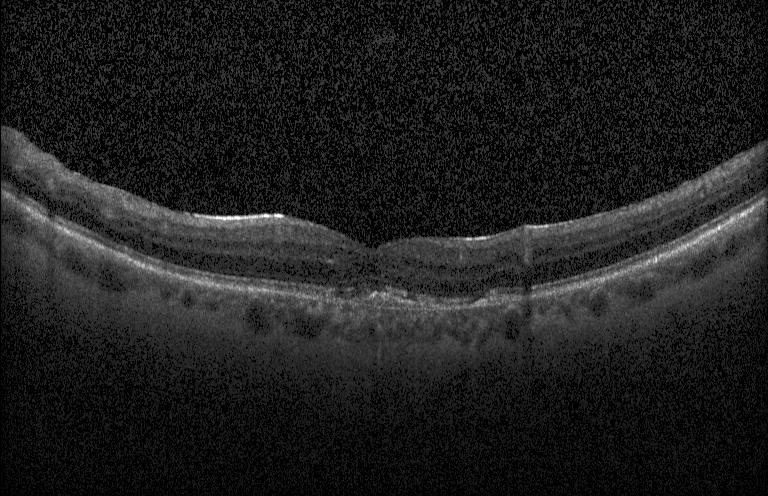 Optical coherence tomography B-scan. Spectral-domain OCT. Instrument: Heidelberg Spectralis. Centered on the fovea.
OCT finding: a choroidal neovascular membrane.